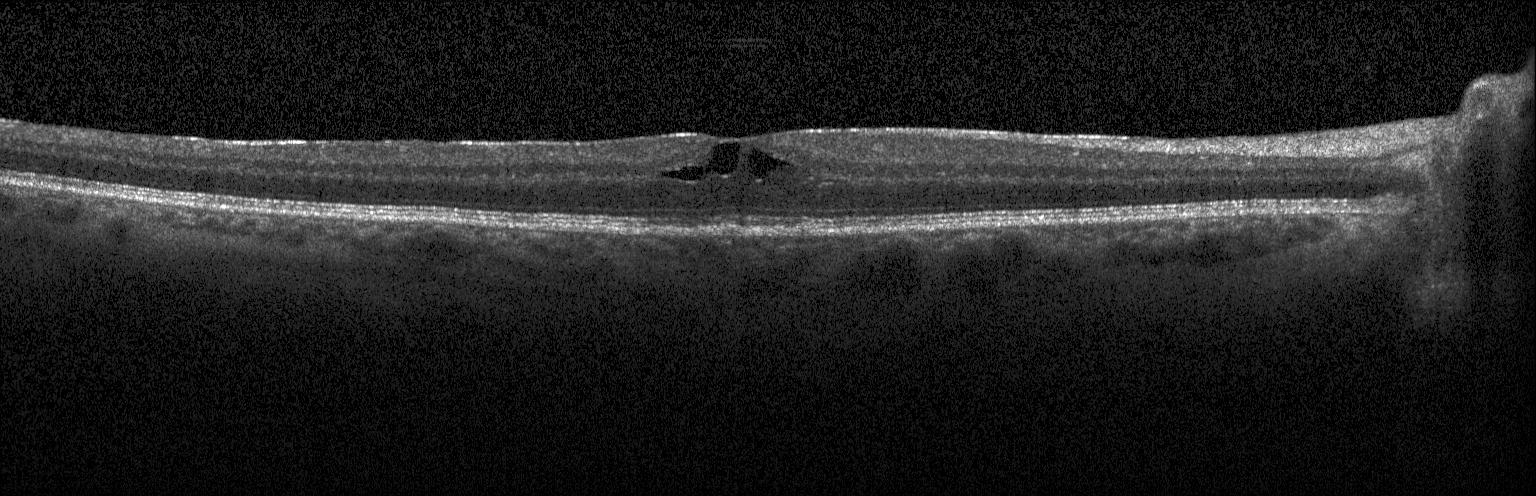
Optical coherence tomography B-scan
Impression: diabetic macular edema.